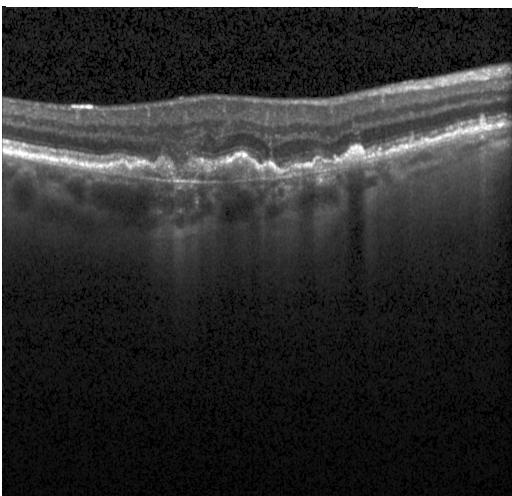
Spectral-domain optical coherence tomography · horizontal scan through the fovea · Heidelberg Spectralis OCT system · OCT B-scan. This B-scan demonstrates CNV.